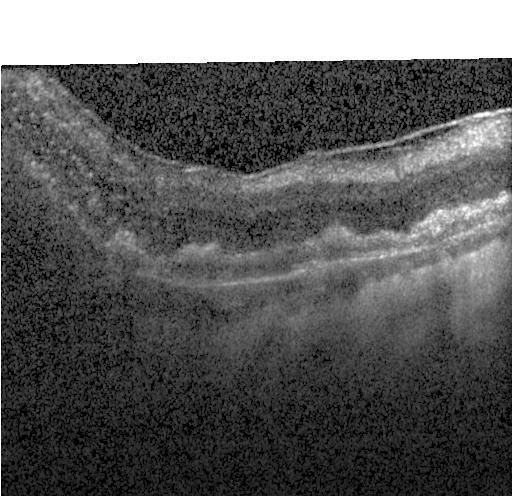

Optical coherence tomography scan.
Diagnosis: CNV.